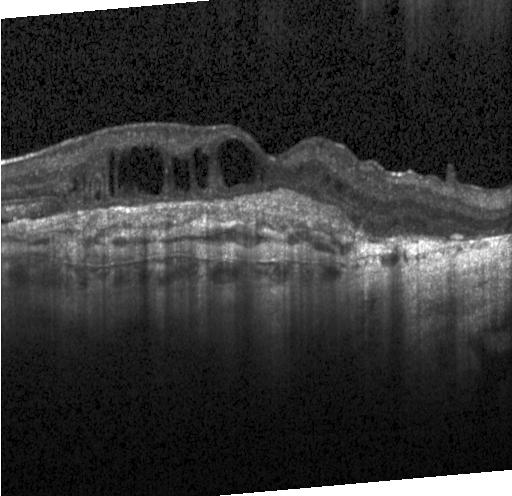

Spectral-domain OCT, macular scan, retinal OCT B-scan. Macular OCT: choroidal neovascularization.